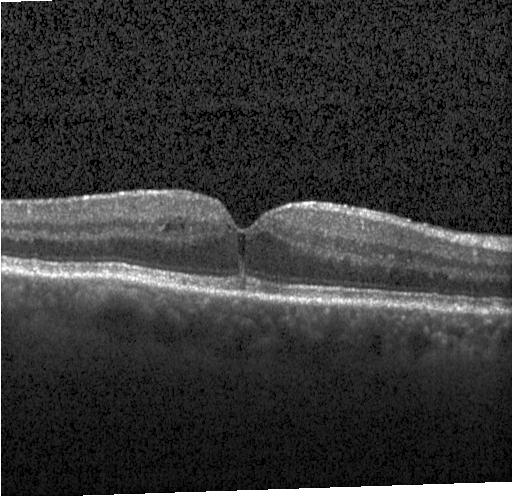
OCT line scan
This B-scan demonstrates DME.